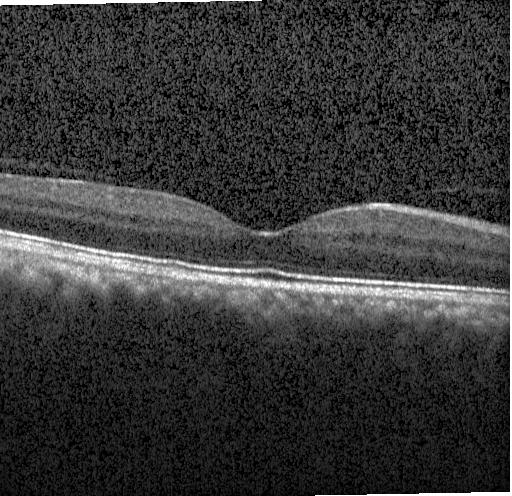
OCT line scan · through the macula · Heidelberg Spectralis OCT system — Assessment: no evidence of choroidal neovascularization, diabetic macular edema, or drusen.